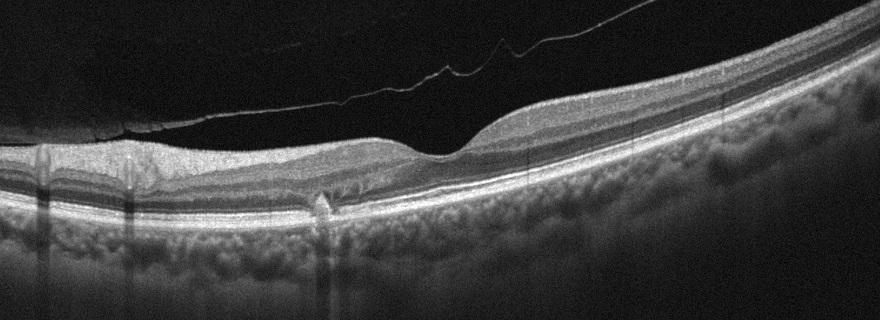

OCT line scan — Diagnosis: AMD.